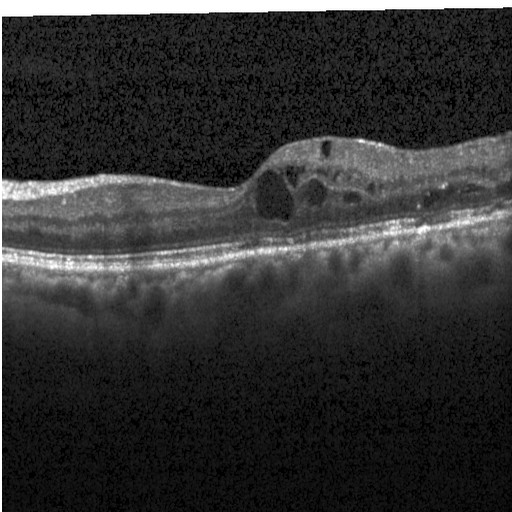

OCT B-scan showing diabetic macular edema.